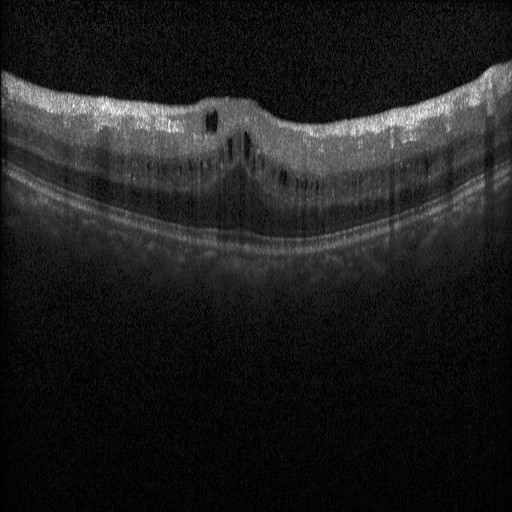 Macular OCT: diabetic macular edema (DME).